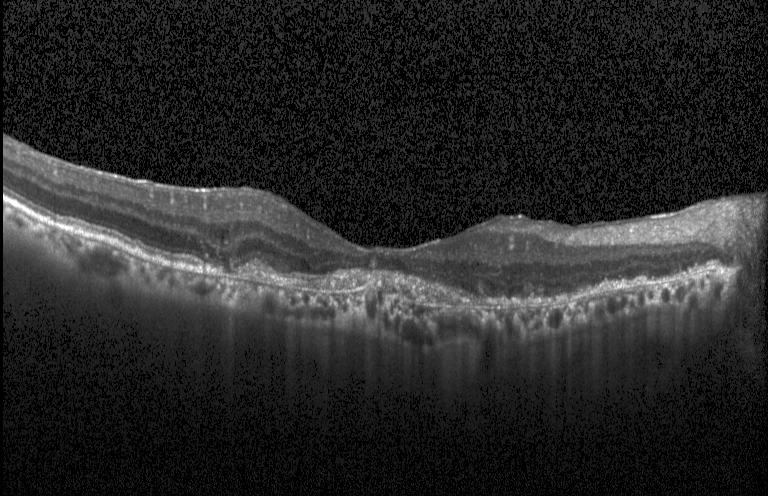 Optical coherence tomography scan. Diagnosis: a choroidal neovascular membrane.